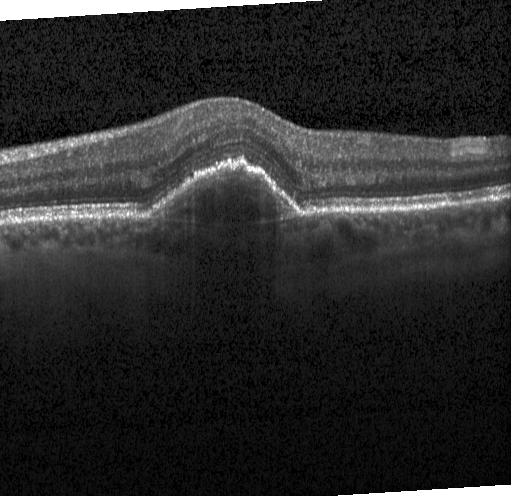 Retinal OCT cross-section.
Assessment: choroidal neovascularization.